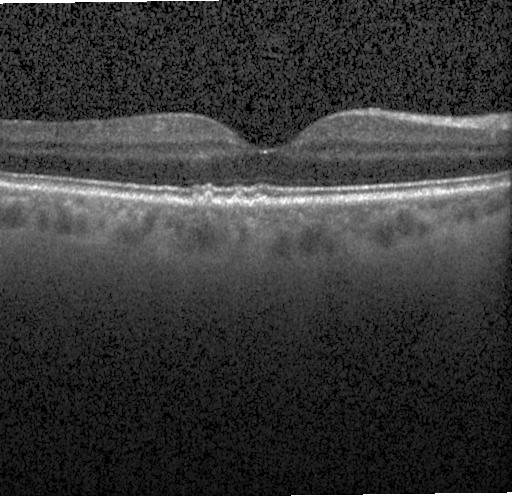
OCT line scan.
Macular OCT: multiple drusen.